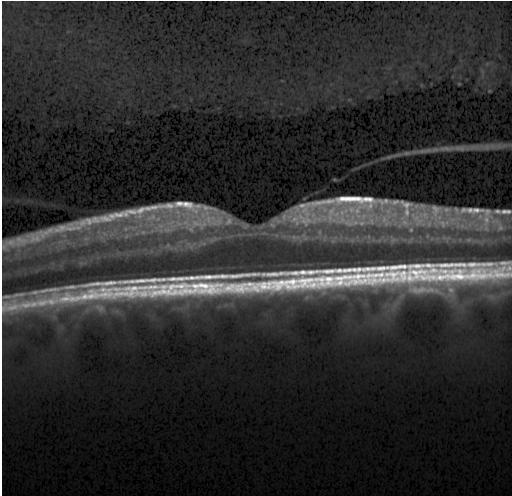
Through the macula; OCT B-scan
Macular OCT: no choroidal neovascularization, no diabetic macular edema, and no drusen.